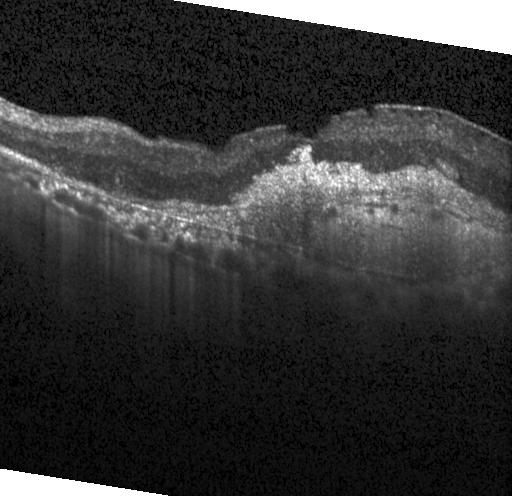

Finding: CNV.